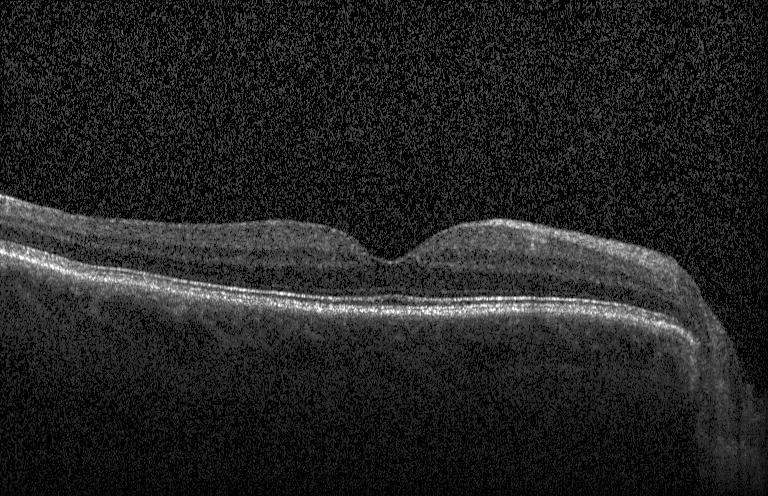

Macular OCT: no evidence of CNV, DME, or drusen.